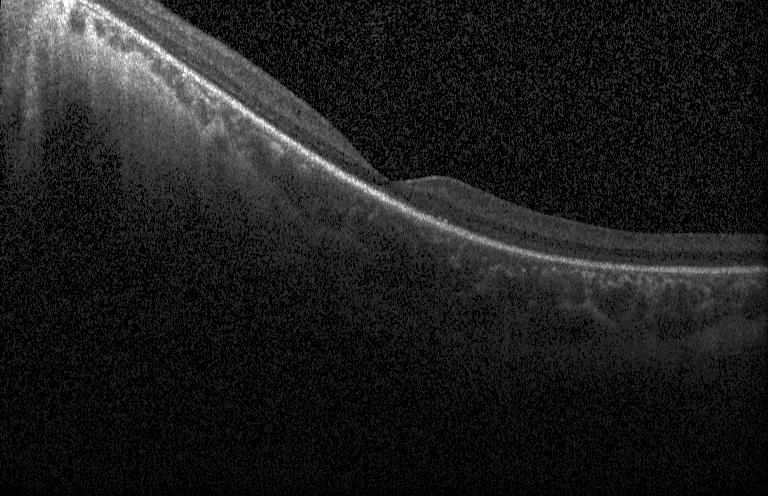
No evidence of choroidal neovascularization, diabetic macular edema, or drusen.